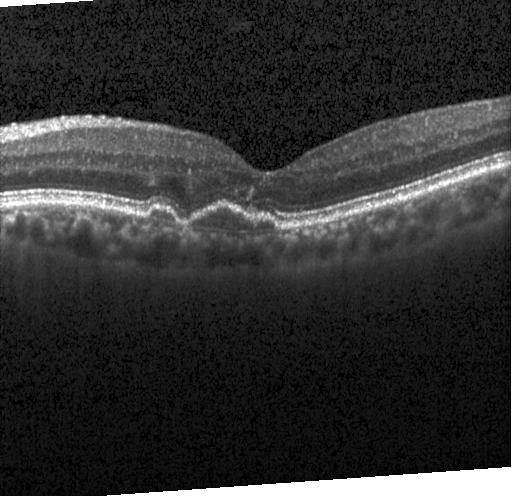 Horizontal scan through the fovea · Heidelberg Spectralis OCT system · optical coherence tomography B-scan. Choroidal neovascularization (CNV).